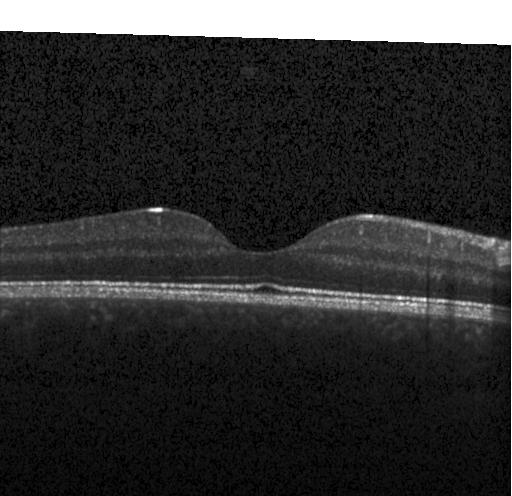 Horizontal scan through the fovea; retinal OCT cross-section; spectral-domain optical coherence tomography
Impression: no CNV, DME, or drusen.